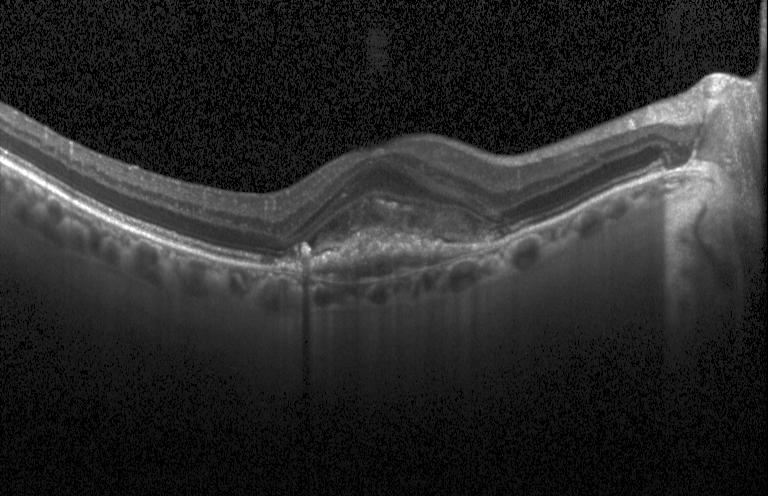

Fovea-centered; OCT B-scan; Heidelberg Spectralis — The scan shows choroidal neovascularization.